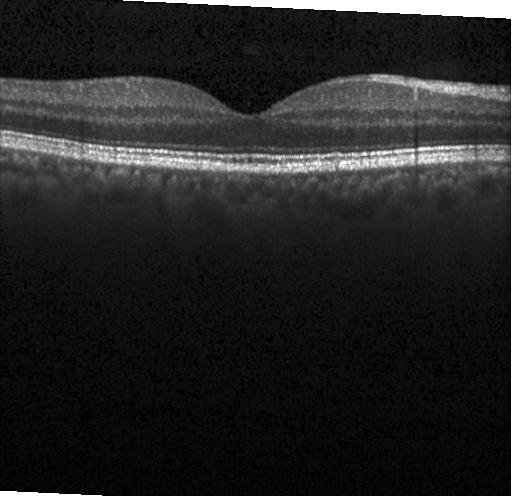 OCT finding: no choroidal neovascularization, diabetic macular edema, or drusen.